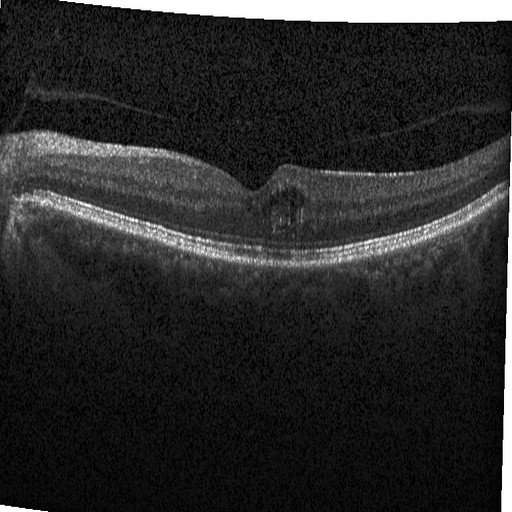 OCT B-scan · SD-OCT · instrument: Heidelberg Spectralis · through the macula. OCT finding: DME.